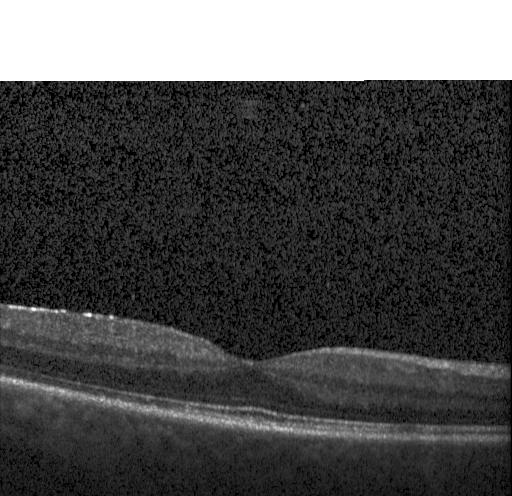 OCT finding: no choroidal neovascularization, diabetic macular edema, or drusen.